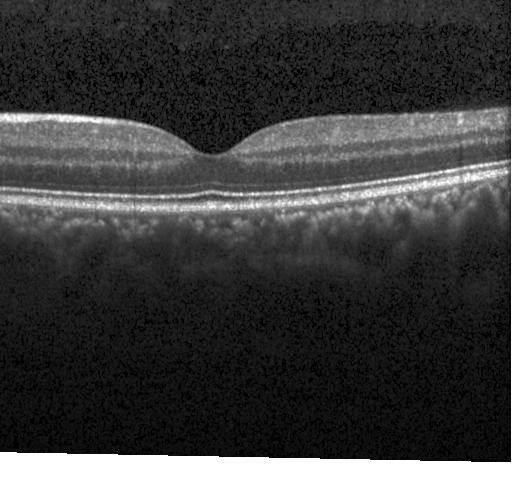

Through the macula, optical coherence tomography scan.
Impression: no evidence of choroidal neovascularization, diabetic macular edema, or drusen.